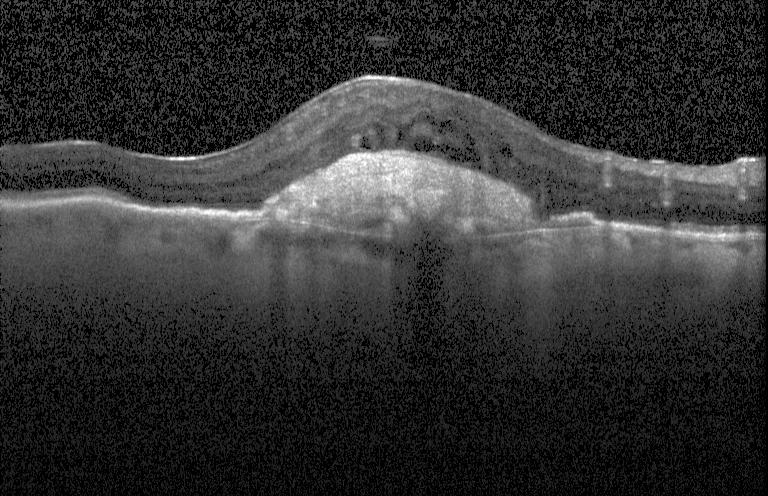

Spectral-domain OCT · retinal OCT cross-section · through the macula.
Finding: choroidal neovascularization.